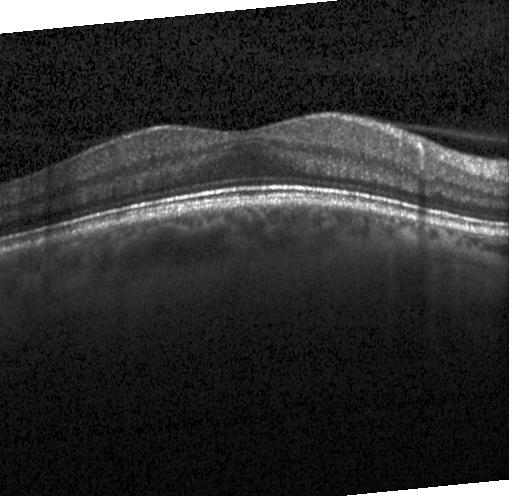

Macular OCT demonstrating no CNV, DME, or drusen.